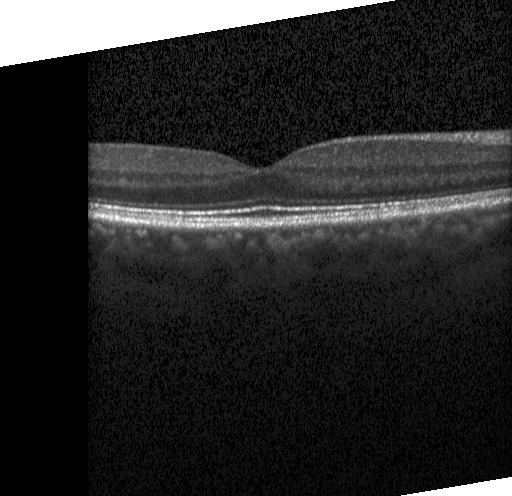
Spectral-domain optical coherence tomography. Centered on the fovea. OCT line scan
Diagnosis: no choroidal neovascularization, diabetic macular edema, or drusen.